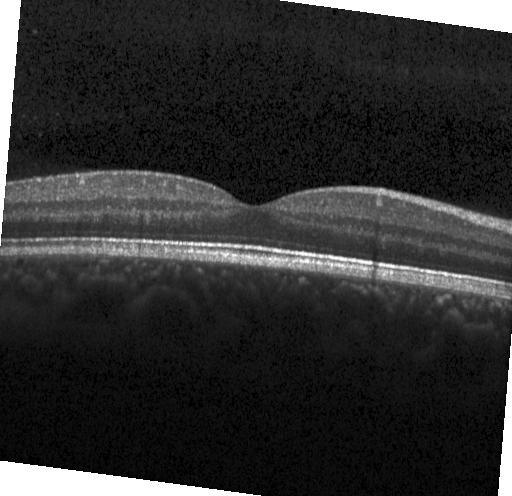
Centered on the fovea; Heidelberg Spectralis OCT system; OCT line scan; spectral-domain OCT
Dx: no evidence of choroidal neovascularization, diabetic macular edema, or drusen.